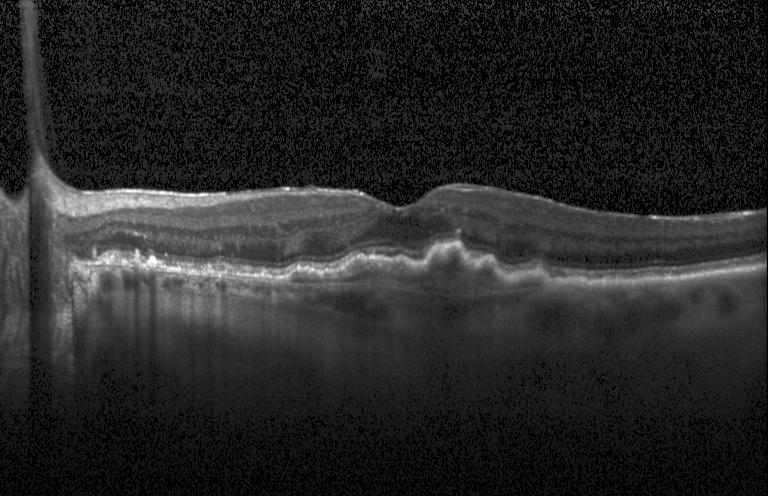 Retinal OCT cross-section — Diagnosis: choroidal neovascularization (CNV).